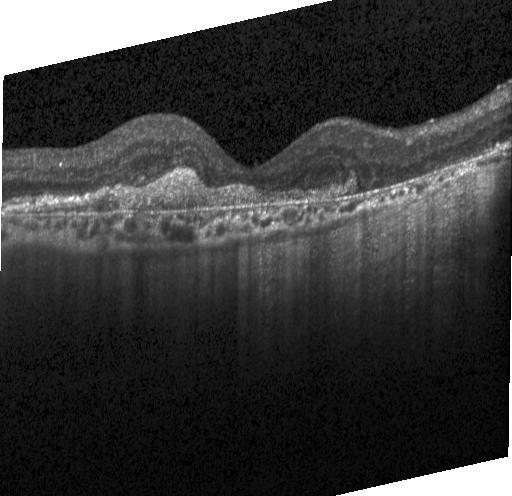
Optical coherence tomography scan. Heidelberg Spectralis OCT system. Spectral-domain optical coherence tomography. Through the macula — A choroidal neovascular membrane.